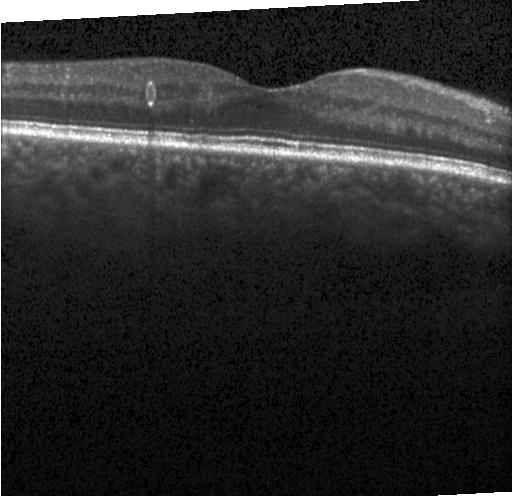 Assessment: no choroidal neovascularization, no diabetic macular edema, and no drusen.